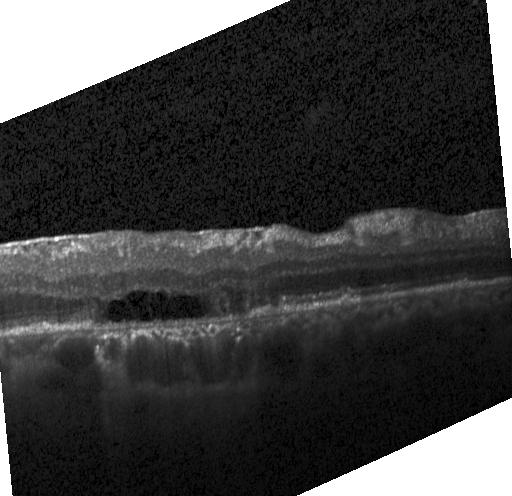

Through the macula. OCT B-scan. Dx: a choroidal neovascular membrane.